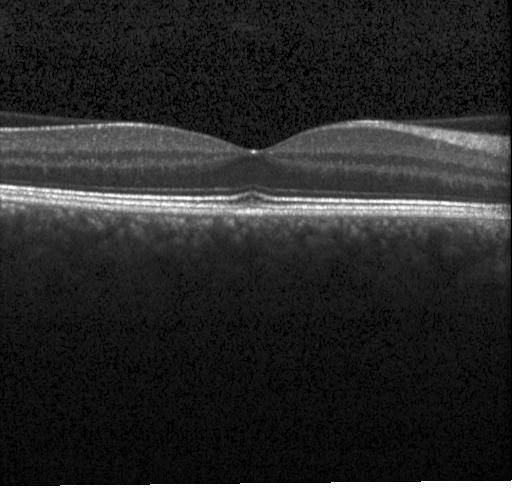
Retinal OCT cross-section.
Assessment: no choroidal neovascularization, no diabetic macular edema, and no drusen.